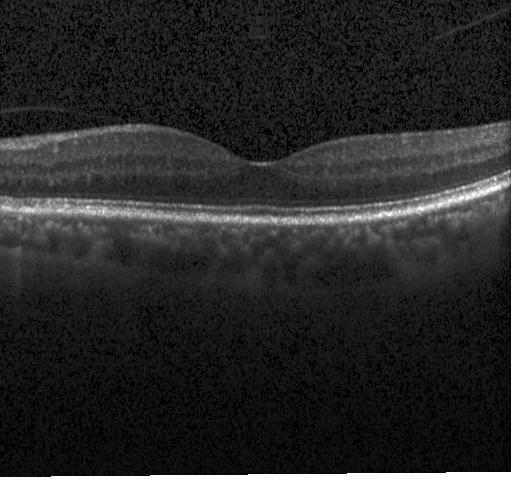

Heidelberg Spectralis · optical coherence tomography B-scan · centered on the fovea.
No evidence of choroidal neovascularization, diabetic macular edema, or drusen.